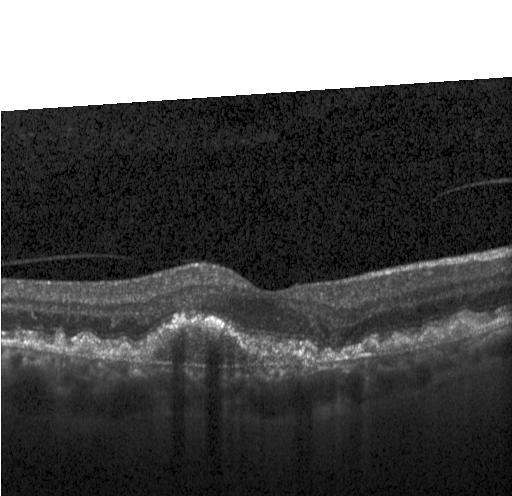

OCT line scan, Heidelberg Spectralis OCT system, spectral-domain optical coherence tomography, through the macula.
Impression: a choroidal neovascular membrane.